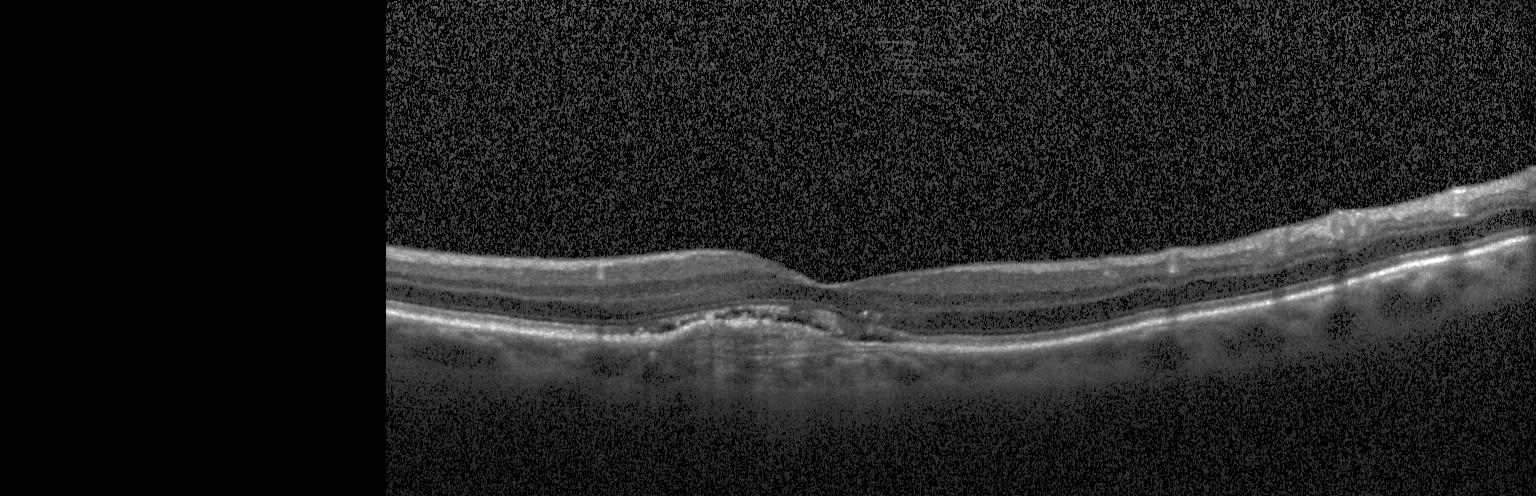

Spectral-domain OCT B-scan: choroidal neovascularization.